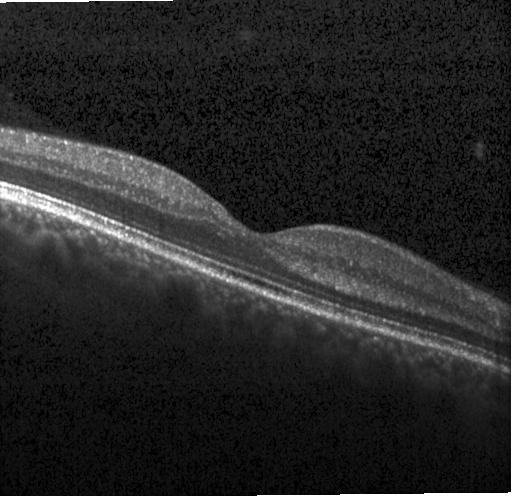

Assessment: neither choroidal neovascularization, diabetic macular edema, nor drusen.